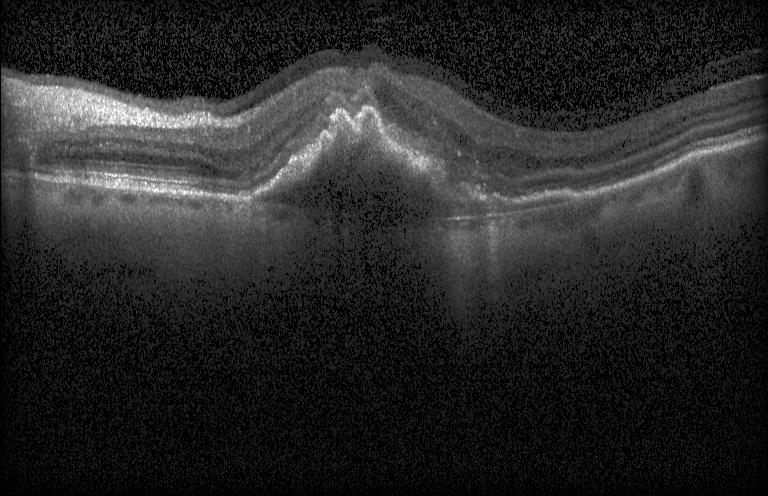

Spectral-domain OCT. Retinal OCT B-scan. Heidelberg Spectralis OCT system. OCT finding: a choroidal neovascular membrane.